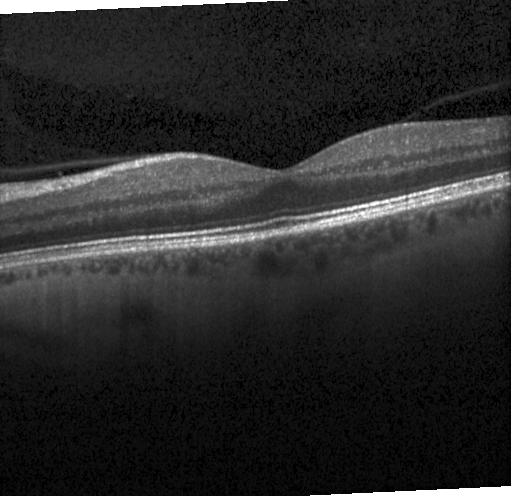

Retinal OCT cross-section; Heidelberg Spectralis OCT system; spectral-domain optical coherence tomography. Finding: neither choroidal neovascularization, diabetic macular edema, nor drusen.